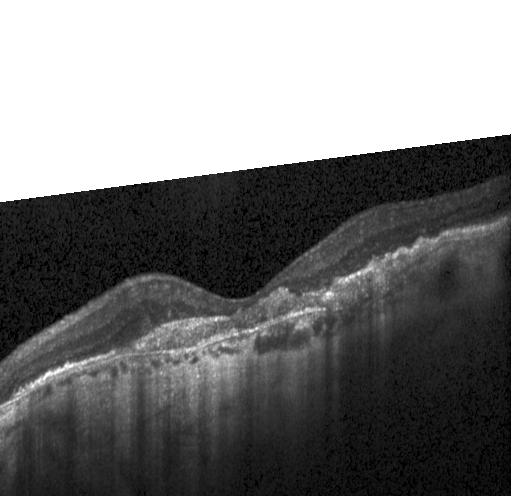 This B-scan demonstrates a choroidal neovascular membrane.